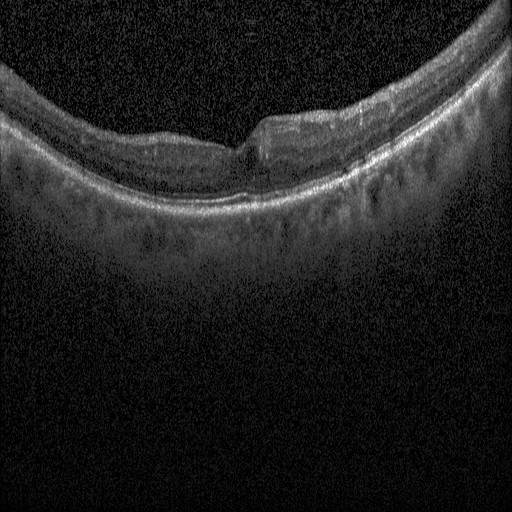

Diagnosis: diabetic macular edema (DME).